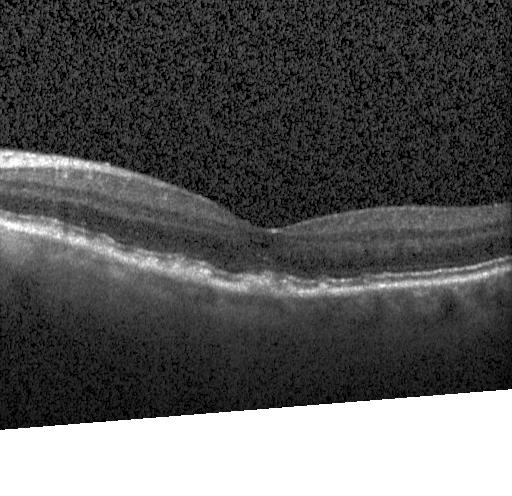 Heidelberg Spectralis; retinal OCT B-scan — Multiple drusen.